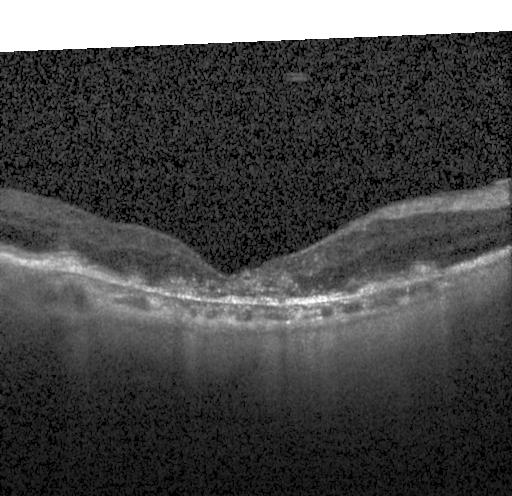
Through the macula, optical coherence tomography B-scan
Finding: a choroidal neovascular membrane.